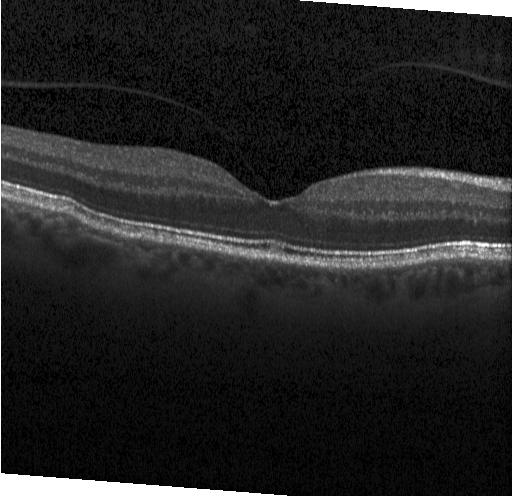
Acquired on a Heidelberg Spectralis; SD-OCT; fovea-centered; retinal OCT cross-section — Impression: no choroidal neovascularization, no diabetic macular edema, and no drusen.